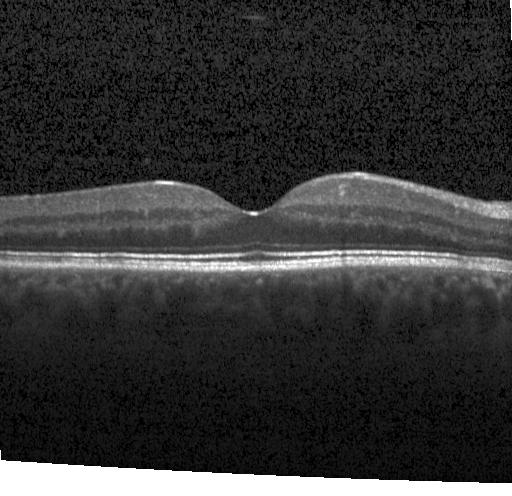 OCT B-scan showing neither CNV, DME, nor drusen.